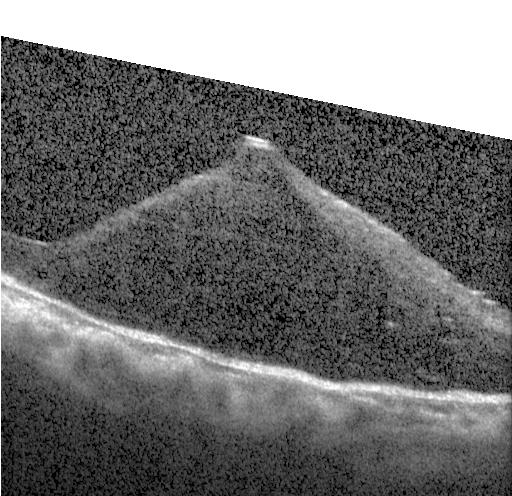
Finding: diabetic macular edema.